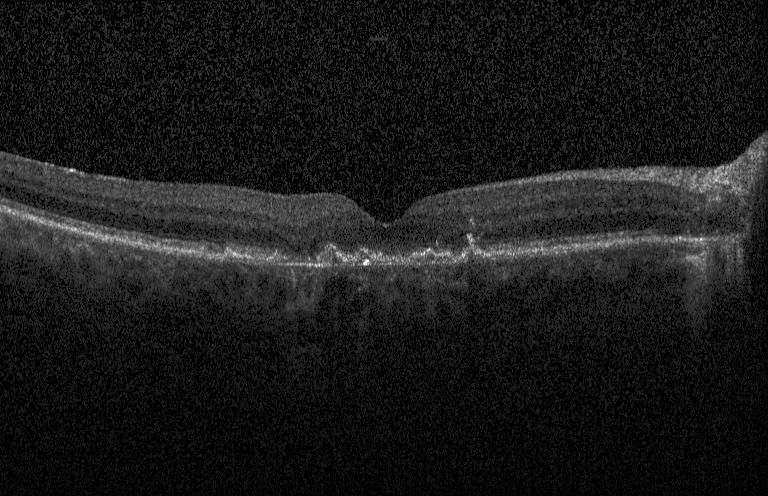 Impression: choroidal neovascularization (CNV).